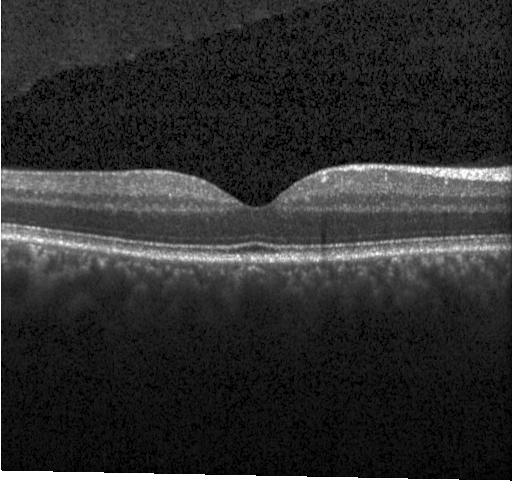
OCT B-scan. Heidelberg Spectralis.
Assessment: neither choroidal neovascularization, diabetic macular edema, nor drusen.